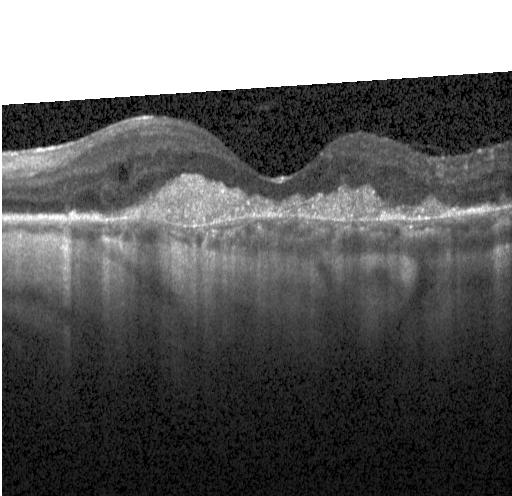

Diagnosis: choroidal neovascularization (CNV).